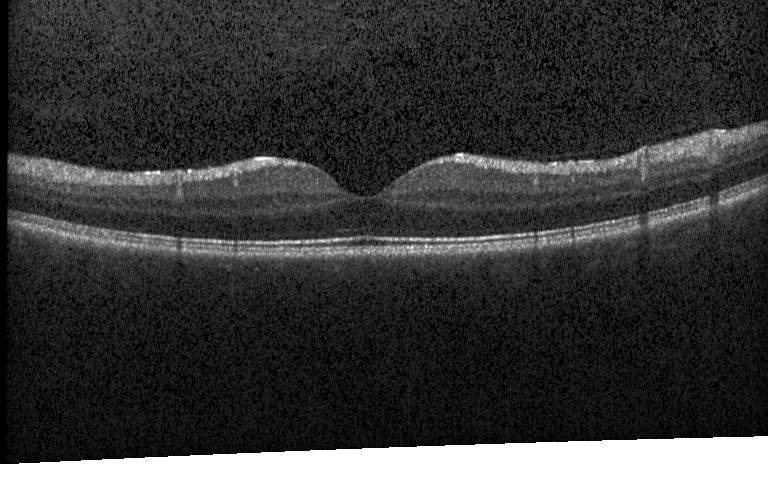 Diagnosis: no choroidal neovascularization, no diabetic macular edema, and no drusen.